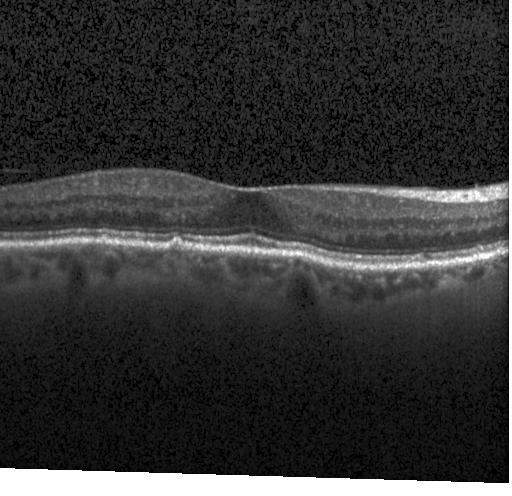
Optical coherence tomography scan; spectral-domain optical coherence tomography.
This B-scan demonstrates drusen.